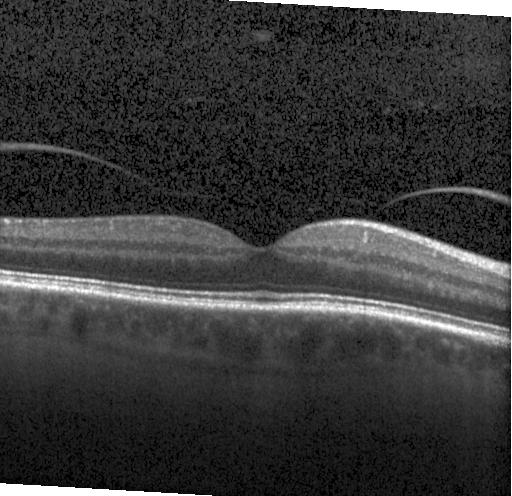 Retinal OCT B-scan. Spectral-domain OCT.
Diagnosis: no CNV, no DME, and no drusen.